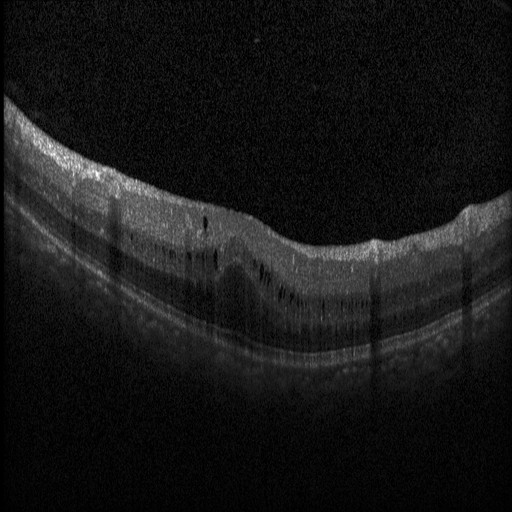 OCT line scan
Finding: diabetic macular edema (DME).